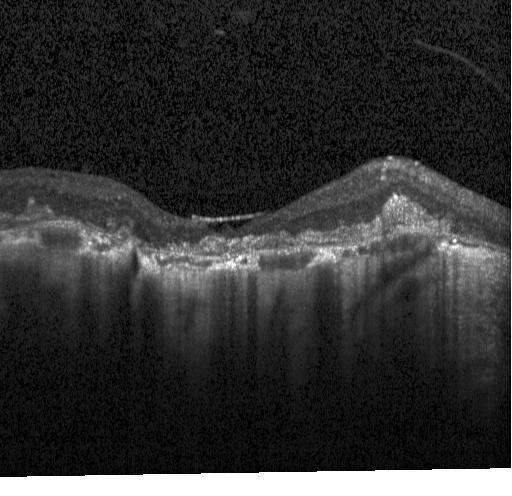 Optical coherence tomography scan. Impression: choroidal neovascularization (CNV).